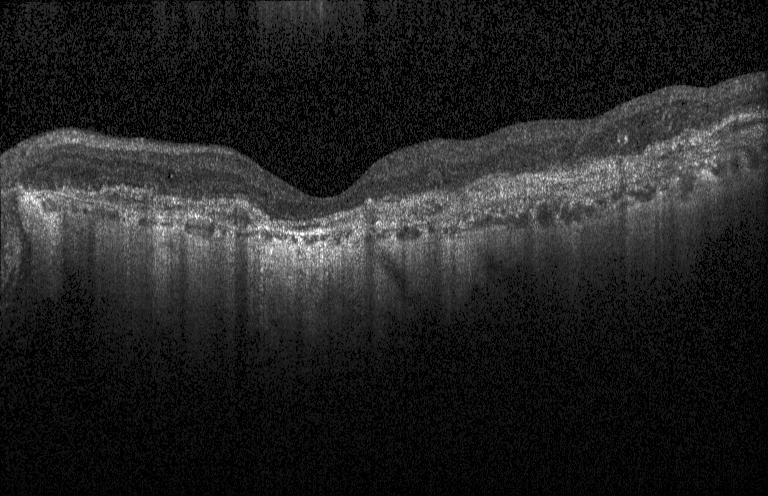
The scan shows a choroidal neovascular membrane.